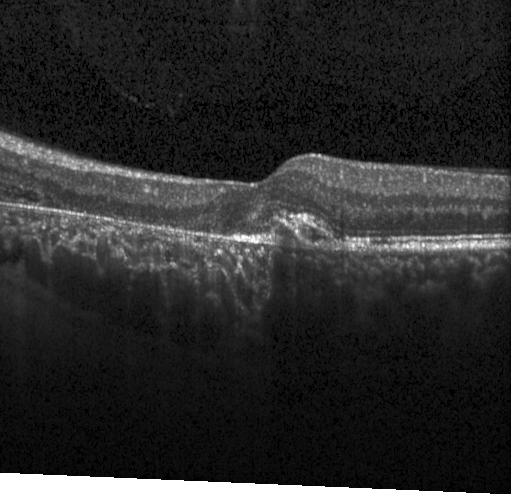 Optical coherence tomography B-scan. Impression: a choroidal neovascular membrane.